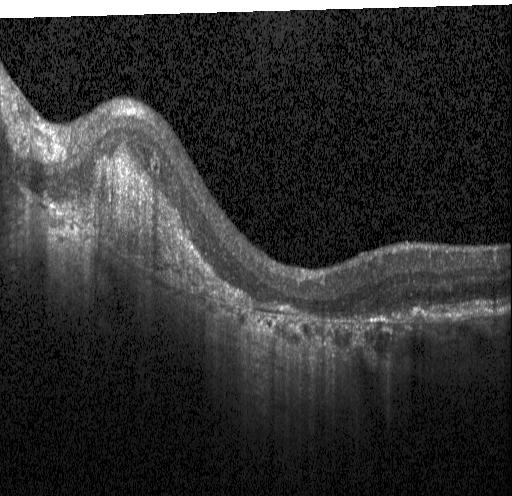 Fovea-centered. Optical coherence tomography scan. Instrument: Heidelberg Spectralis. OCT finding: choroidal neovascularization.